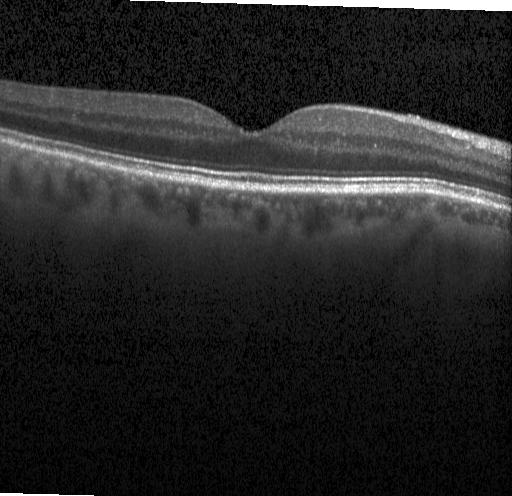
OCT finding: no evidence of CNV, DME, or drusen.